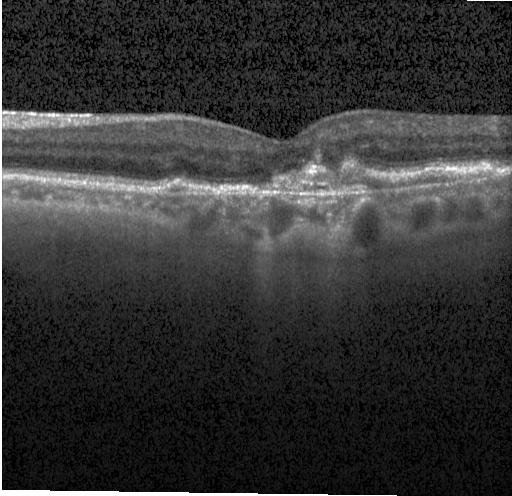

Optical coherence tomography scan. Centered on the fovea. Spectral-domain OCT. Heidelberg Spectralis. Diagnosis: CNV.